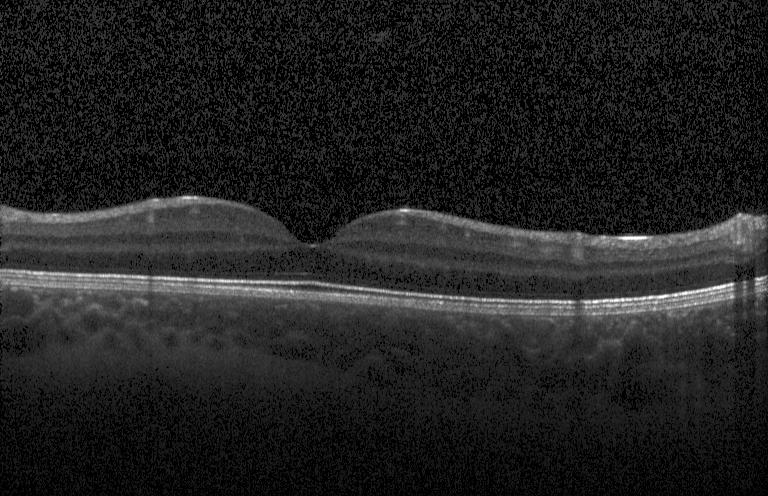 Centered on the fovea. Optical coherence tomography scan. Heidelberg Spectralis. SD-OCT.
Diagnosis: no choroidal neovascularization, diabetic macular edema, or drusen.